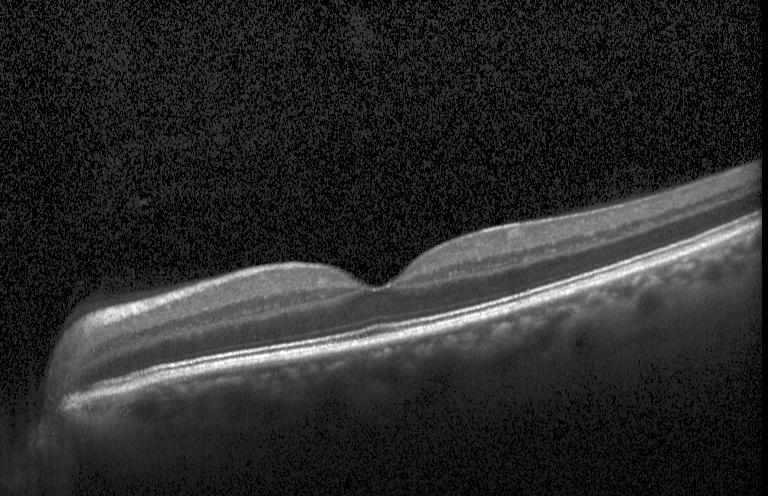
The scan shows no choroidal neovascularization, no diabetic macular edema, and no drusen.